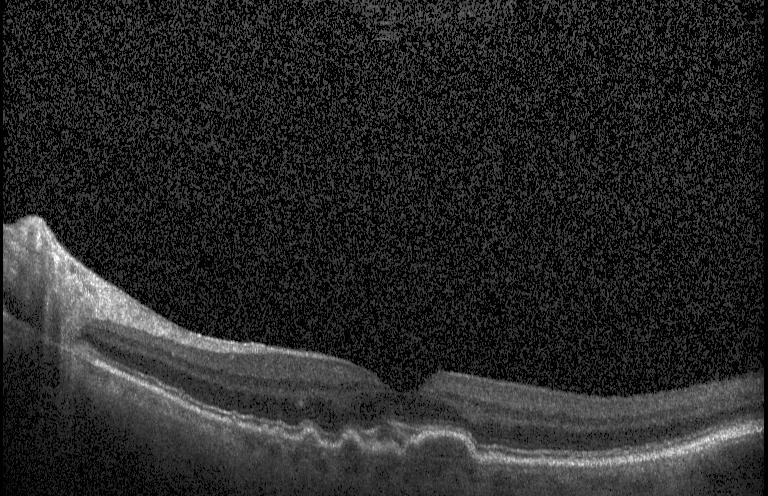
Retinal OCT B-scan.
Impression: drusen.